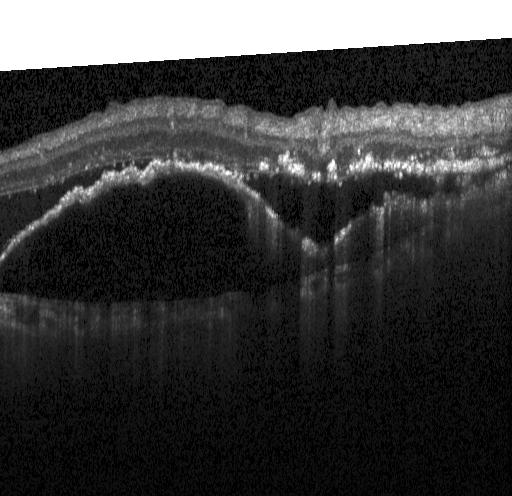

Dx: choroidal neovascularization (CNV).